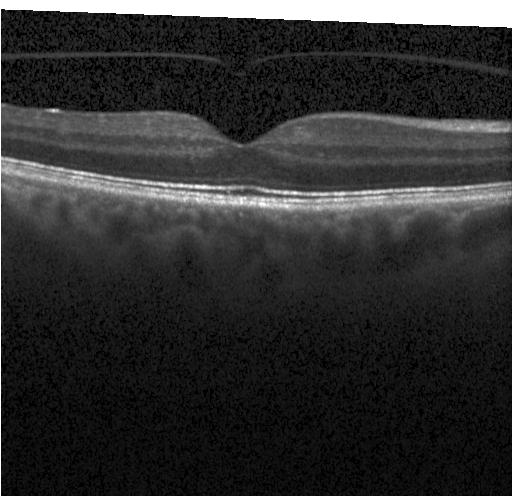

OCT line scan, spectral-domain OCT, centered on the fovea, instrument: Heidelberg Spectralis — Diagnosis: no evidence of choroidal neovascularization, diabetic macular edema, or drusen.